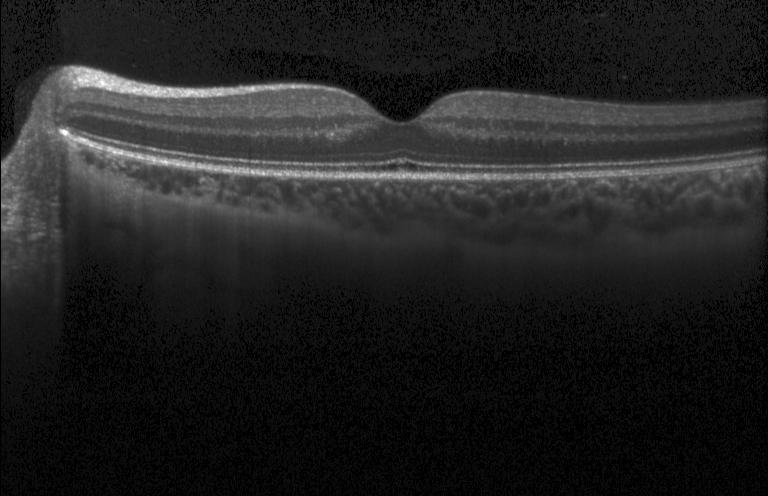
Retinal OCT B-scan · through the macula · acquired on a Heidelberg Spectralis · spectral-domain optical coherence tomography — Assessment: neither choroidal neovascularization, diabetic macular edema, nor drusen.